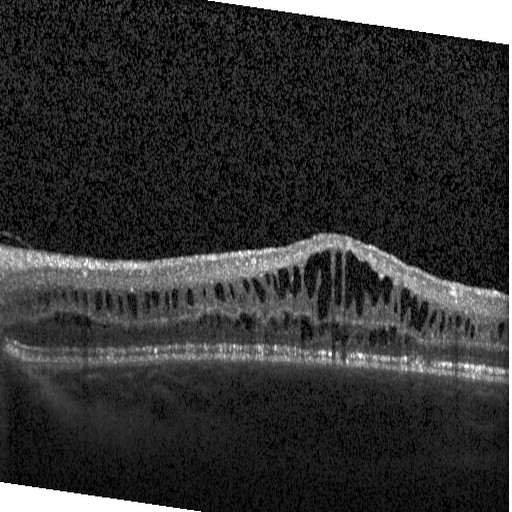
Macular OCT: diabetic macular edema.